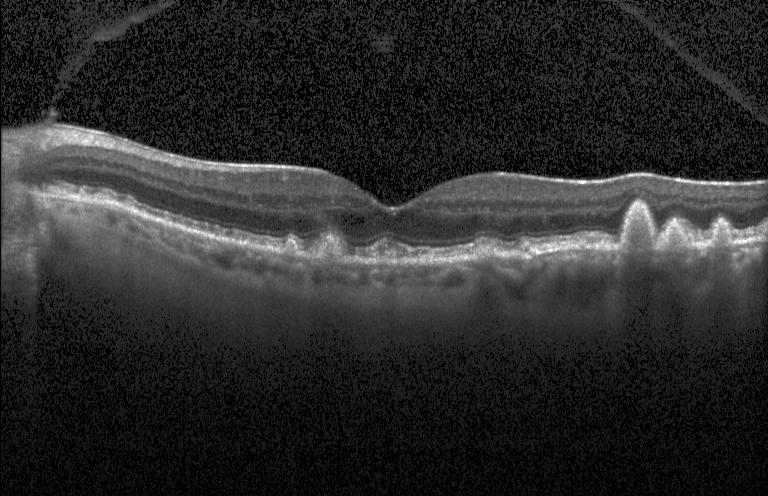
Heidelberg Spectralis · optical coherence tomography B-scan · horizontal scan through the fovea.
Impression: a choroidal neovascular membrane.